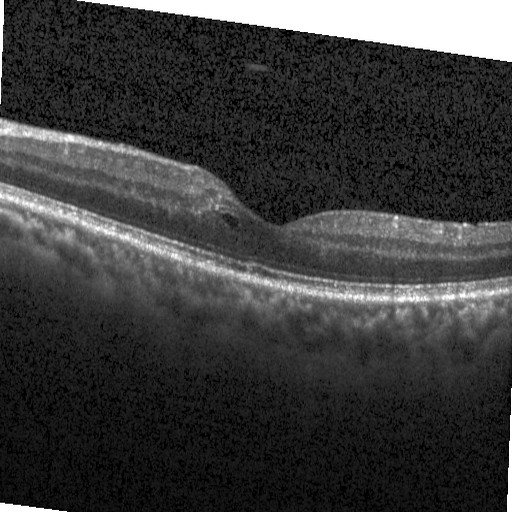 Optical coherence tomography B-scan. Through the macula. Heidelberg Spectralis OCT system. Spectral-domain OCT
Impression: diabetic macular edema (DME).